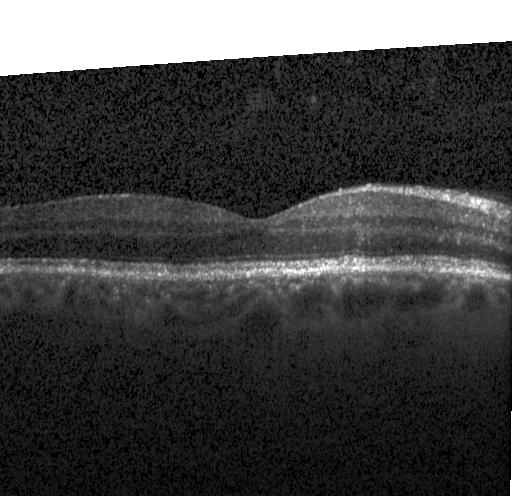

Optical coherence tomography B-scan; acquired on a Heidelberg Spectralis; through the macula; spectral-domain OCT — The scan shows neither CNV, DME, nor drusen.